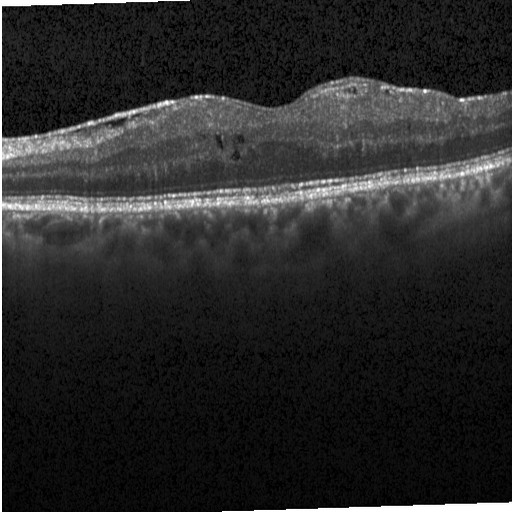 OCT B-scan; Heidelberg Spectralis OCT system — Macular OCT: diabetic macular edema.